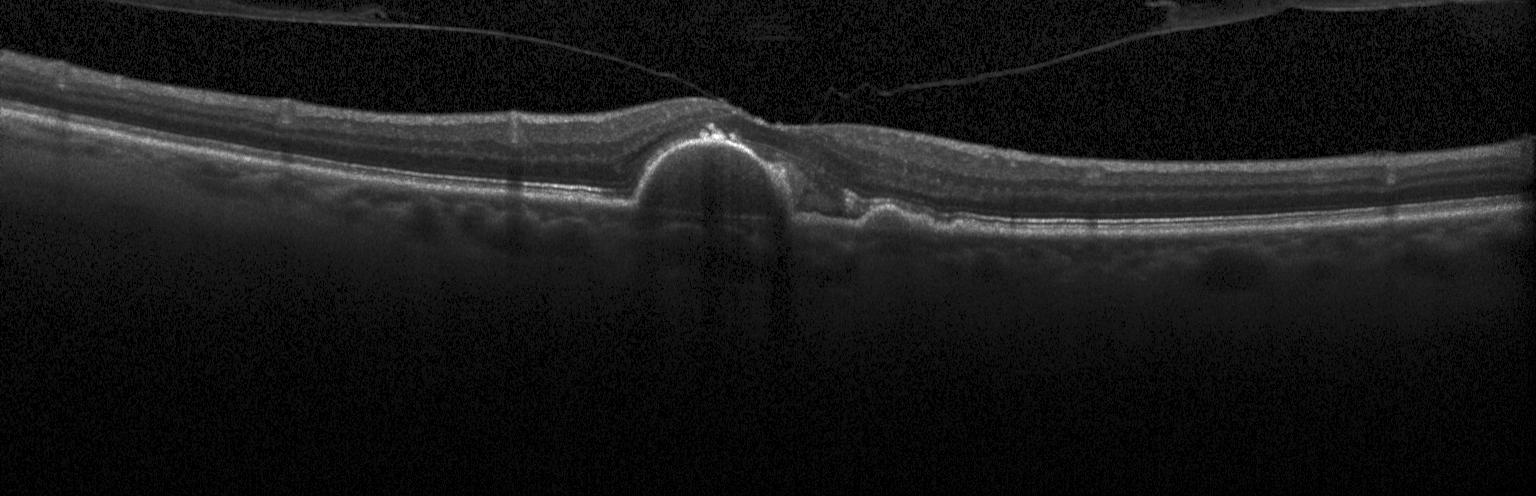

Impression: a choroidal neovascular membrane.